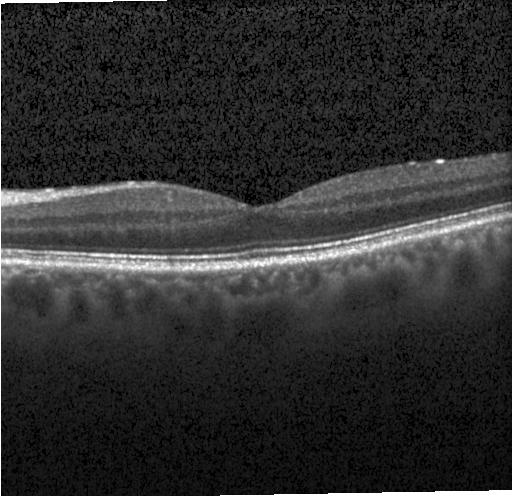 Acquired on a Heidelberg Spectralis; retinal OCT cross-section; fovea-centered; spectral-domain OCT. This B-scan demonstrates no choroidal neovascularization, diabetic macular edema, or drusen.